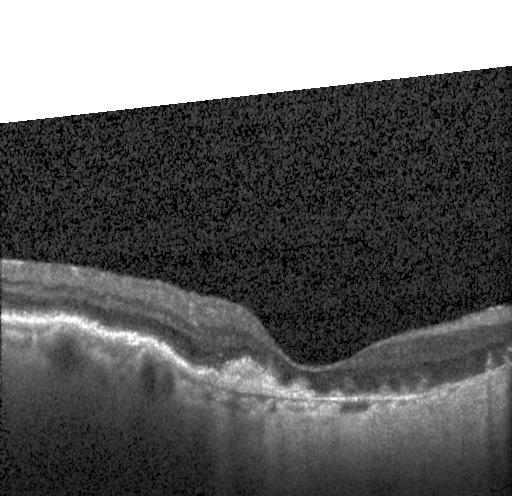

Retinal OCT B-scan. Through the macula.
Finding: CNV.